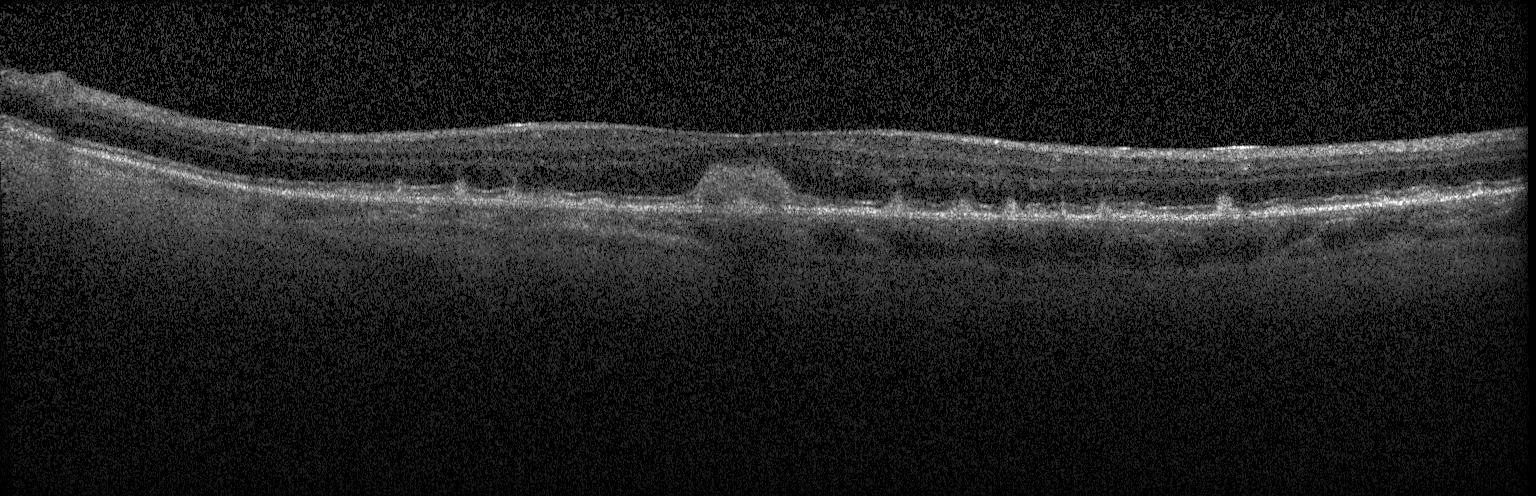 Macular scan, spectral-domain optical coherence tomography, retinal OCT cross-section, Heidelberg Spectralis OCT system
Impression: choroidal neovascularization (CNV).